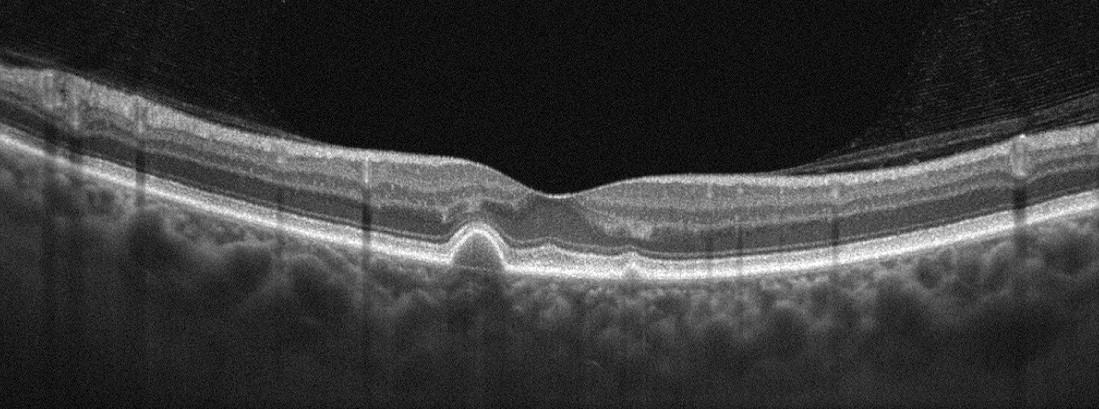

Macular scan. OCT line scan. Impression: AMD.